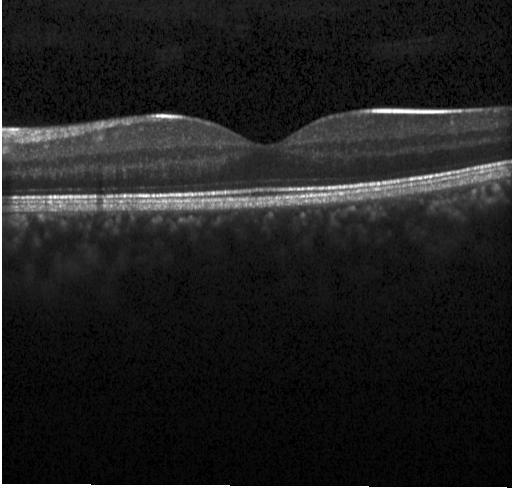
Macular OCT demonstrating neither CNV, DME, nor drusen.